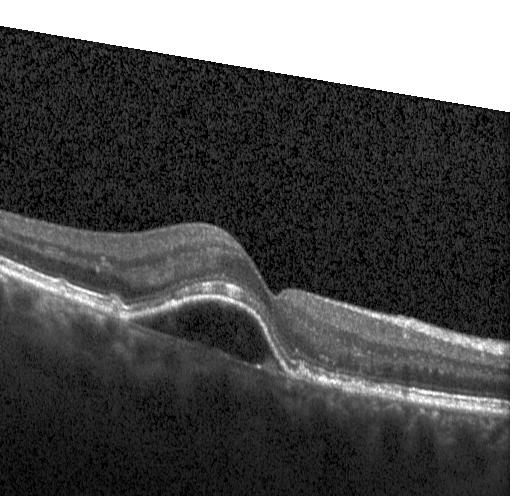 OCT B-scan · horizontal scan through the fovea · acquired on a Heidelberg Spectralis — OCT finding: a choroidal neovascular membrane.